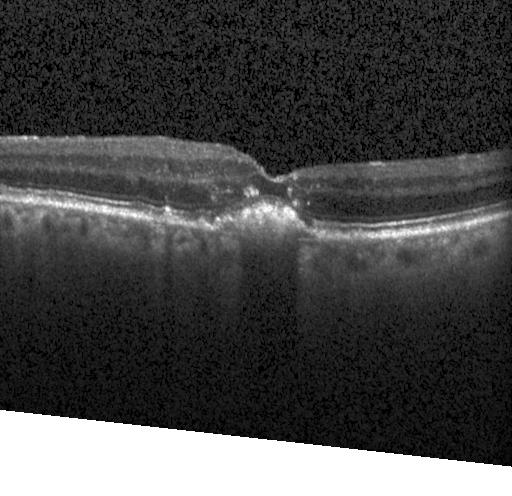
Heidelberg Spectralis · optical coherence tomography B-scan · SD-OCT — Assessment: choroidal neovascularization (CNV).